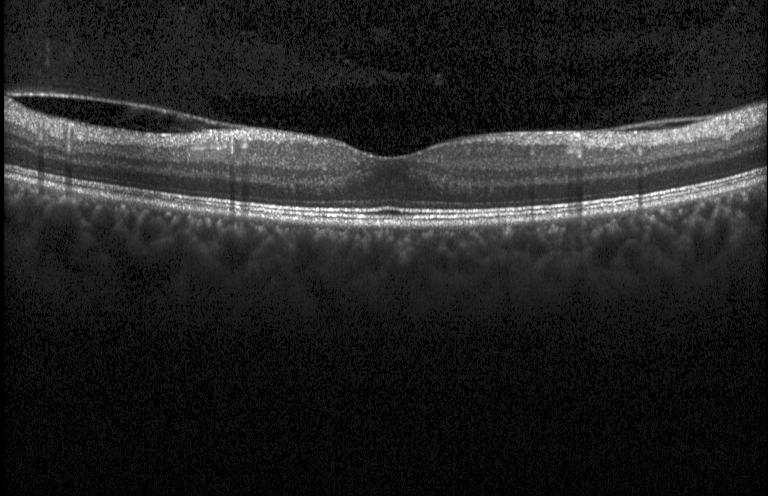

Through the macula, optical coherence tomography B-scan, Heidelberg Spectralis OCT system, spectral-domain optical coherence tomography. Assessment: no choroidal neovascularization, diabetic macular edema, or drusen.